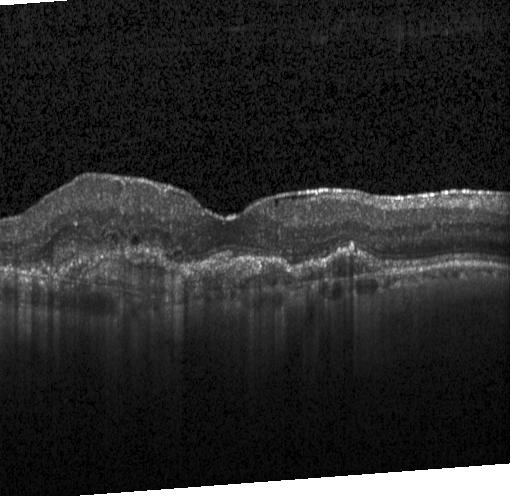

Retinal OCT B-scan
Finding: a choroidal neovascular membrane.